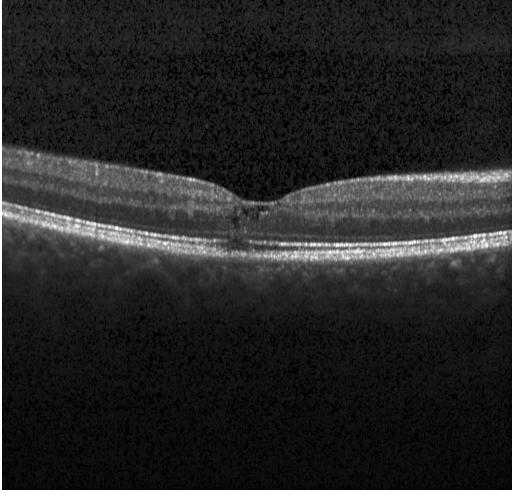
OCT B-scan, instrument: Heidelberg Spectralis, spectral-domain OCT, macular scan — Finding: DME.